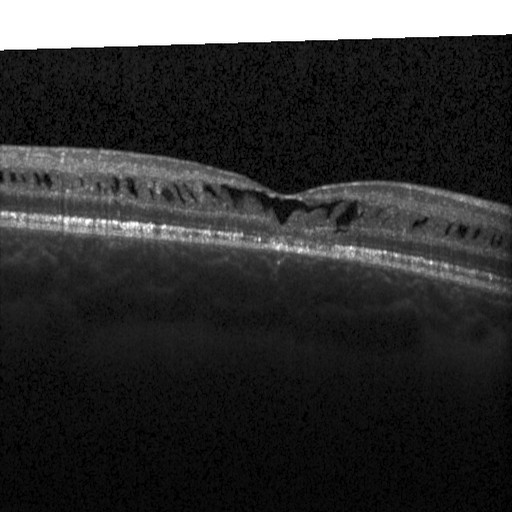

OCT line scan — Impression: diabetic macular edema (DME).